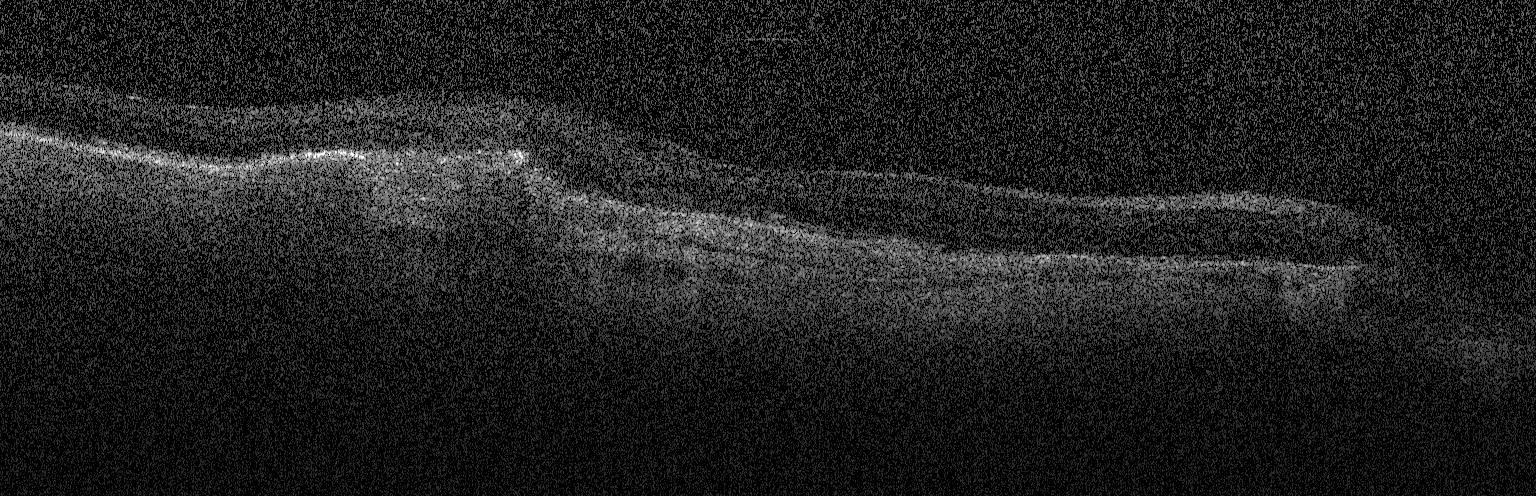 Retinal OCT cross-section · Heidelberg Spectralis OCT system — Finding: choroidal neovascularization (CNV).